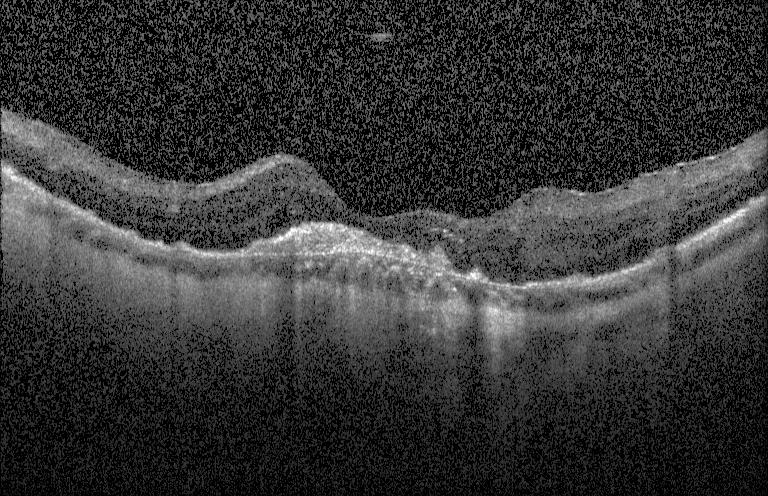

SD-OCT; retinal OCT B-scan.
Diagnosis: a choroidal neovascular membrane.